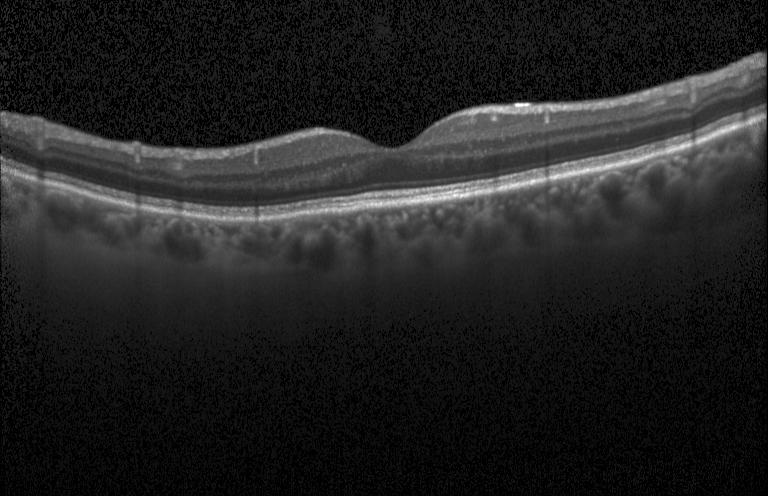
Diagnosis: neither CNV, DME, nor drusen.